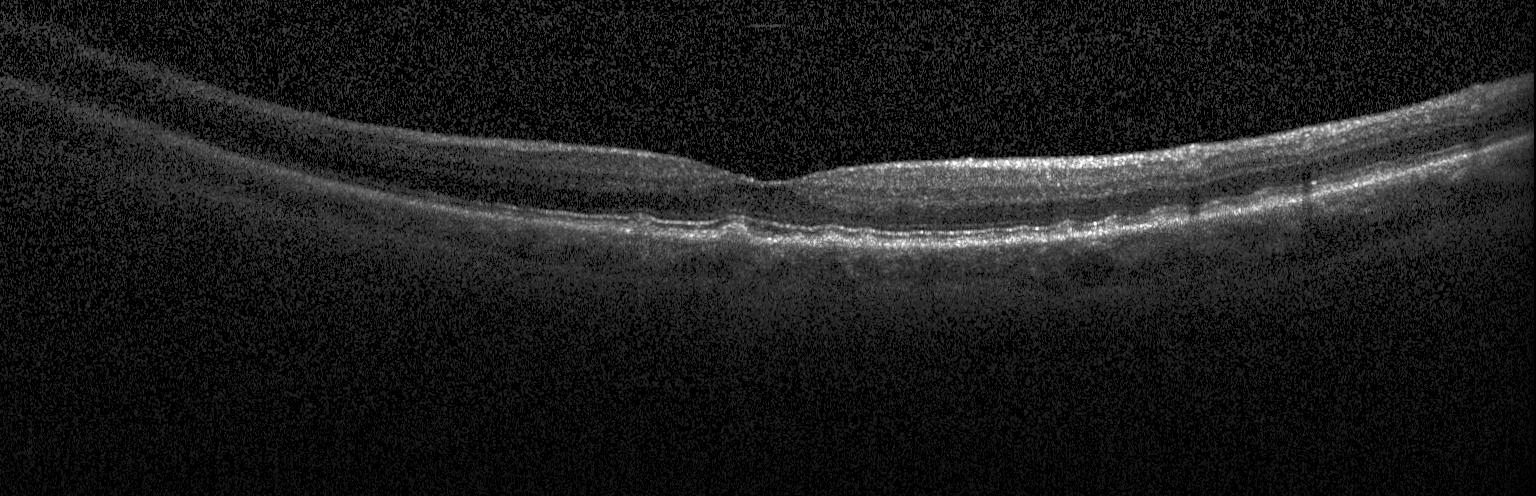 Heidelberg Spectralis · OCT B-scan · SD-OCT.
Dx: sub-RPE drusenoid deposits.